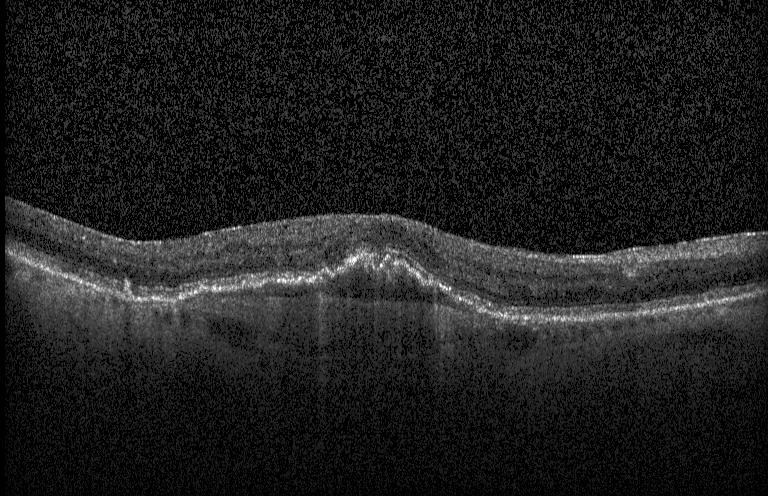

Fovea-centered; Heidelberg Spectralis OCT system; SD-OCT; optical coherence tomography scan
Impression: a choroidal neovascular membrane.